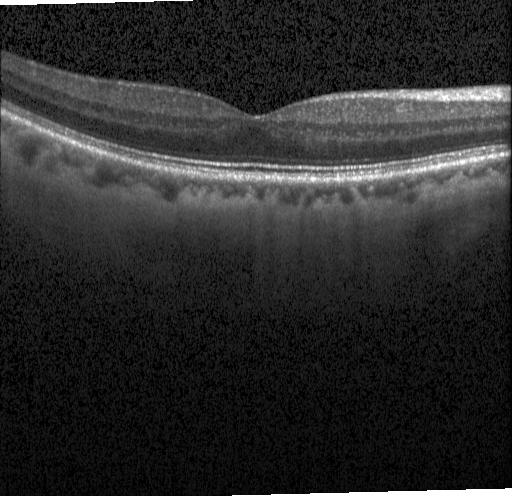

OCT B-scan showing no CNV, no DME, and no drusen.